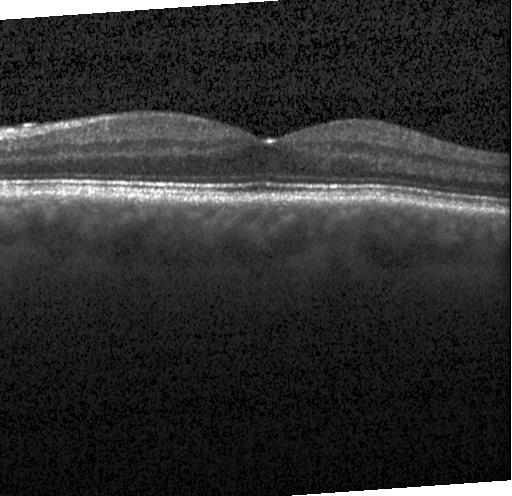

Assessment: no evidence of choroidal neovascularization, diabetic macular edema, or drusen.